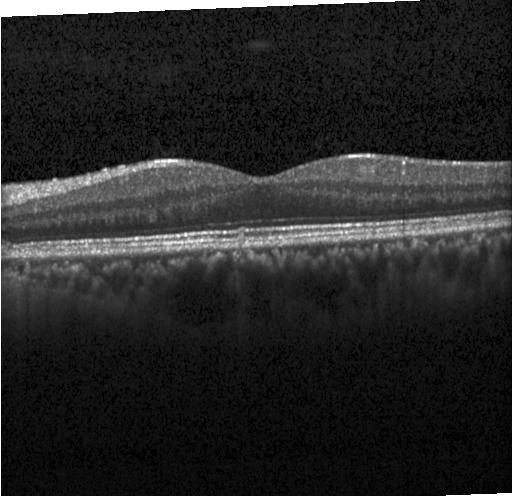
Spectral-domain OCT. OCT line scan — OCT finding: no choroidal neovascularization, diabetic macular edema, or drusen.